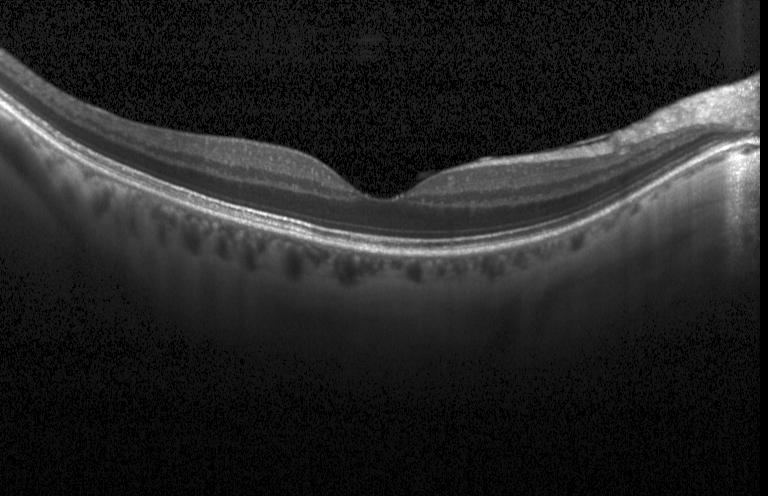 SD-OCT. Retinal OCT B-scan. Instrument: Heidelberg Spectralis
Finding: neither CNV, DME, nor drusen.